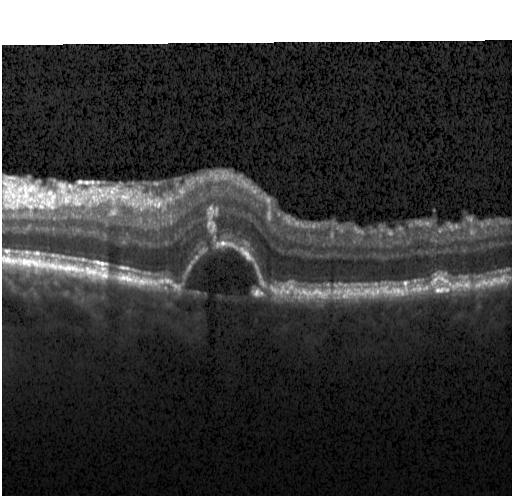
Diagnosis: a choroidal neovascular membrane.